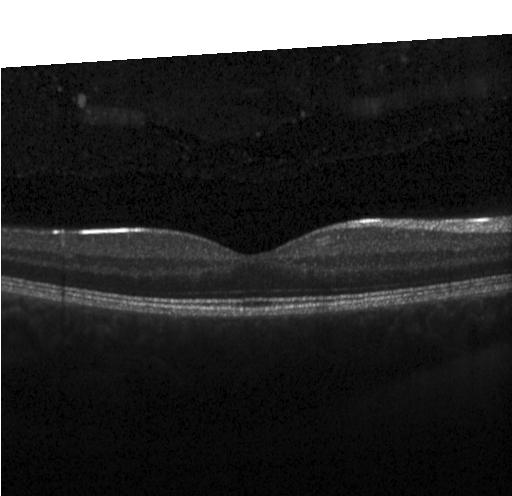 OCT line scan; Heidelberg Spectralis; fovea-centered; spectral-domain optical coherence tomography. The scan shows neither CNV, DME, nor drusen.